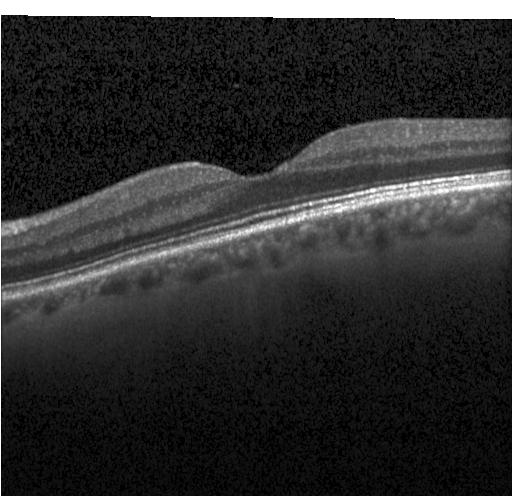 OCT B-scan · macular scan · spectral-domain OCT.
No CNV, no DME, and no drusen.